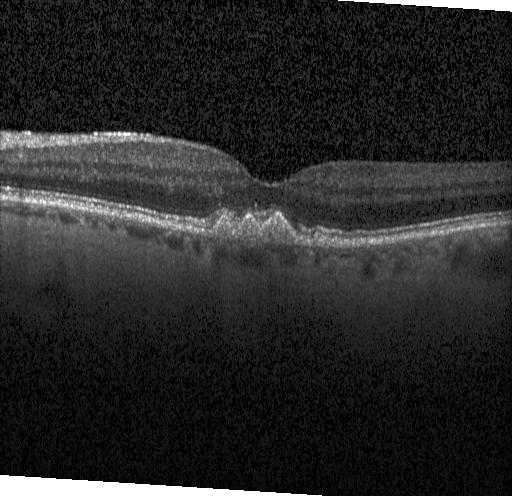 Optical coherence tomography B-scan; SD-OCT; Heidelberg Spectralis OCT system
Assessment: sub-RPE drusenoid deposits.